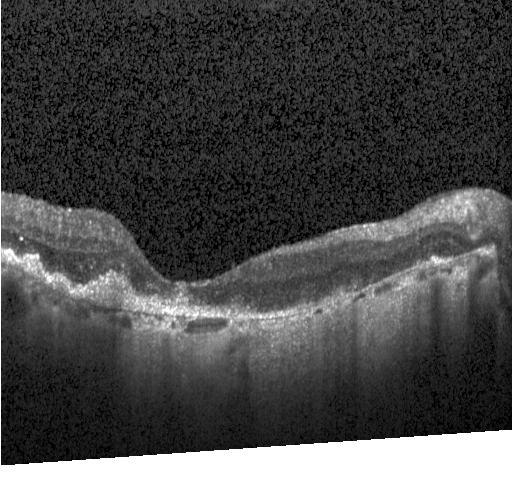
Heidelberg Spectralis OCT system; macular scan; optical coherence tomography B-scan; spectral-domain optical coherence tomography — Impression: a choroidal neovascular membrane.